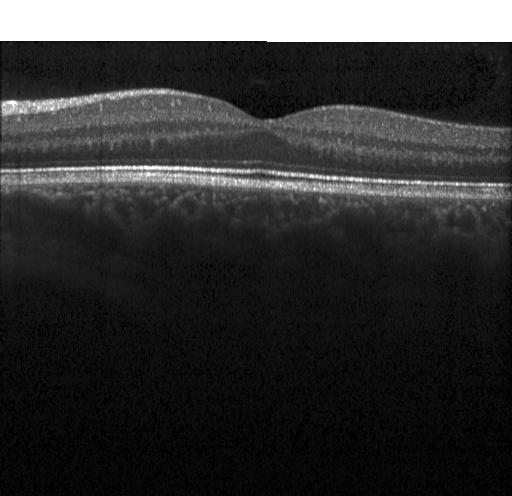
Optical coherence tomography scan — Macular OCT: no evidence of CNV, DME, or drusen.